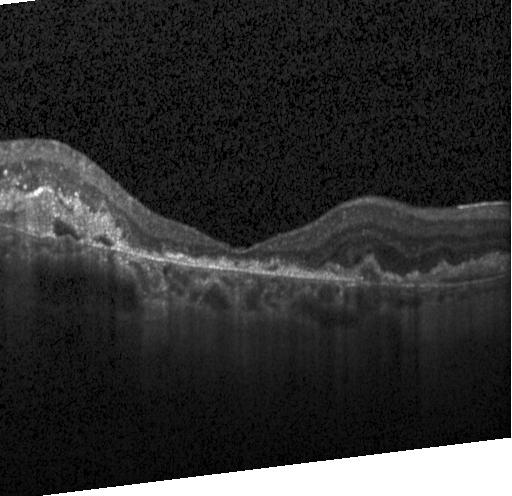

Diagnosis: CNV.